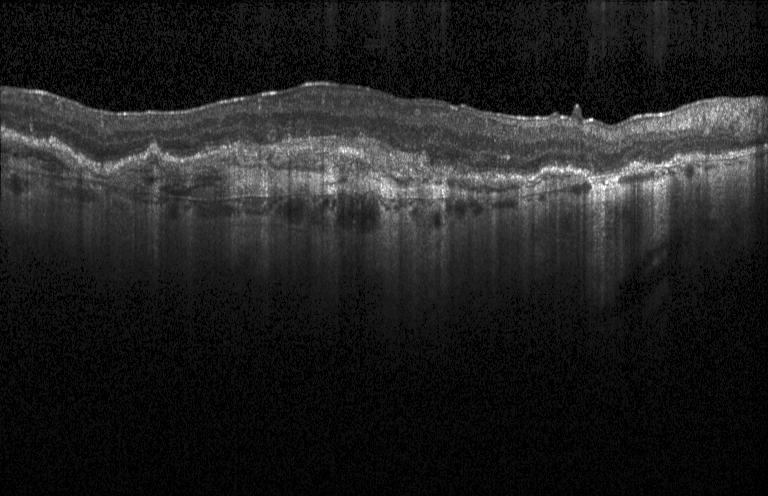 Spectral-domain OCT B-scan: a choroidal neovascular membrane.